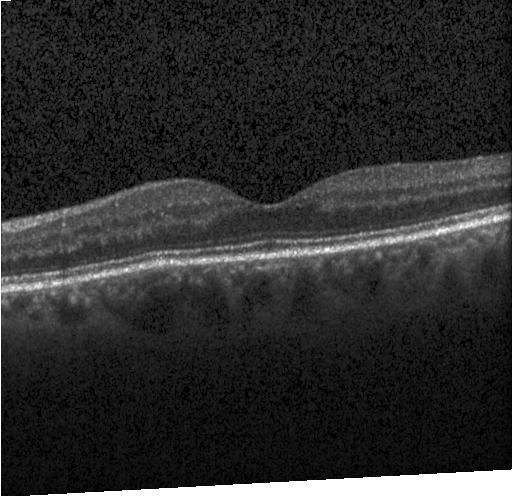 Heidelberg Spectralis OCT system. OCT B-scan. No evidence of choroidal neovascularization, diabetic macular edema, or drusen.